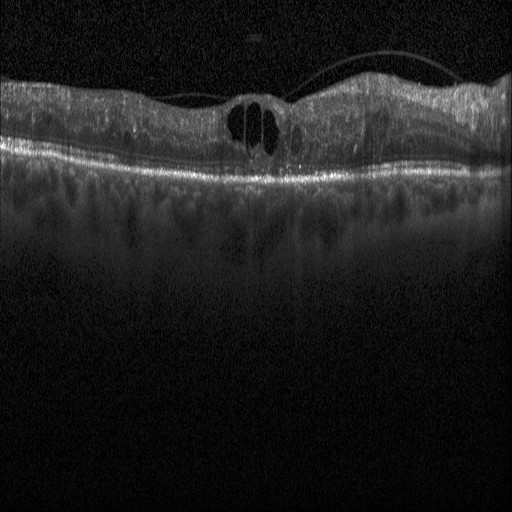
Heidelberg Spectralis OCT system, through the macula, retinal OCT cross-section, spectral-domain OCT — This B-scan demonstrates diabetic macular edema.